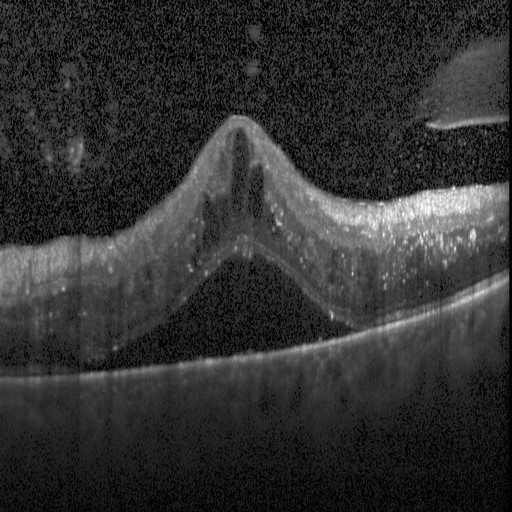

Retinal OCT B-scan — Impression: DME.